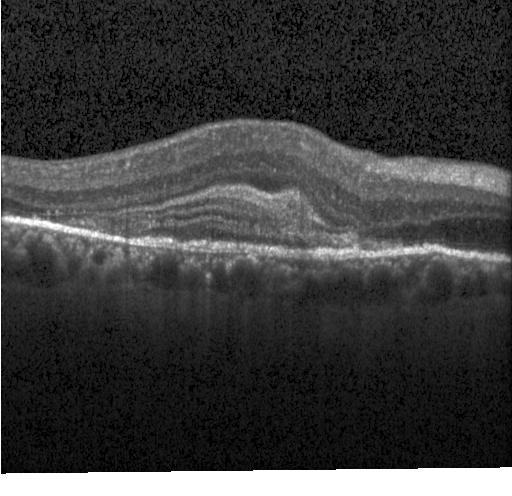

This B-scan demonstrates choroidal neovascularization.